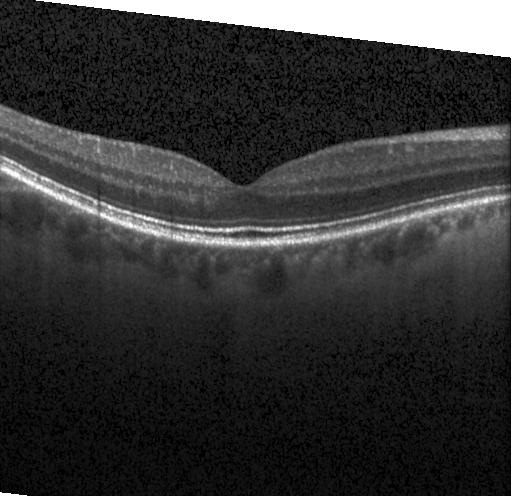 Retinal OCT B-scan — Finding: neither choroidal neovascularization, diabetic macular edema, nor drusen.